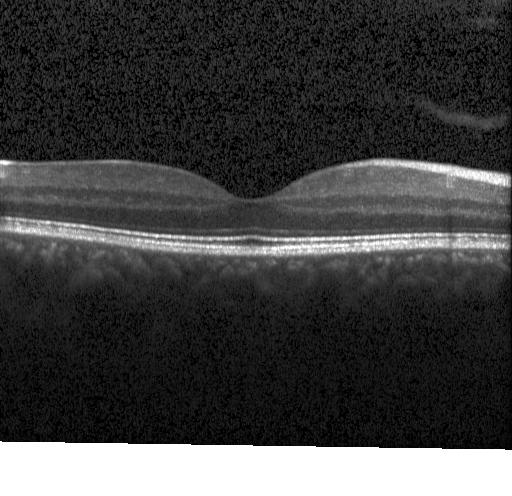 Diagnosis: neither choroidal neovascularization, diabetic macular edema, nor drusen.